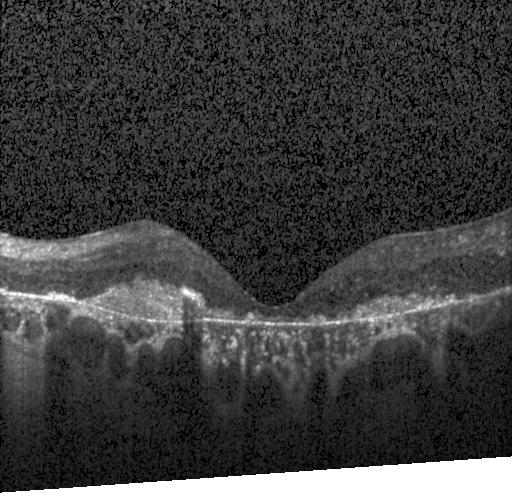
OCT B-scan showing a choroidal neovascular membrane.